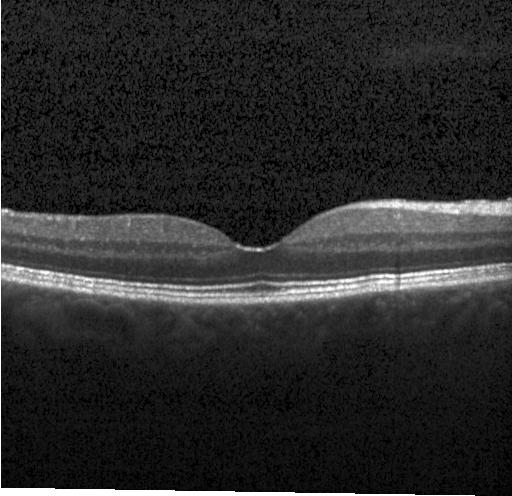
Diagnosis: no evidence of choroidal neovascularization, diabetic macular edema, or drusen.